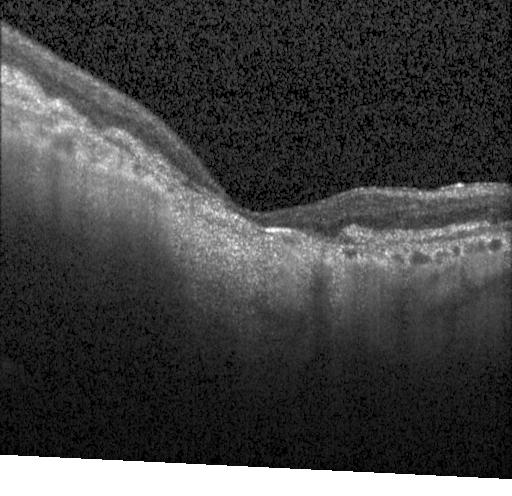
CNV.